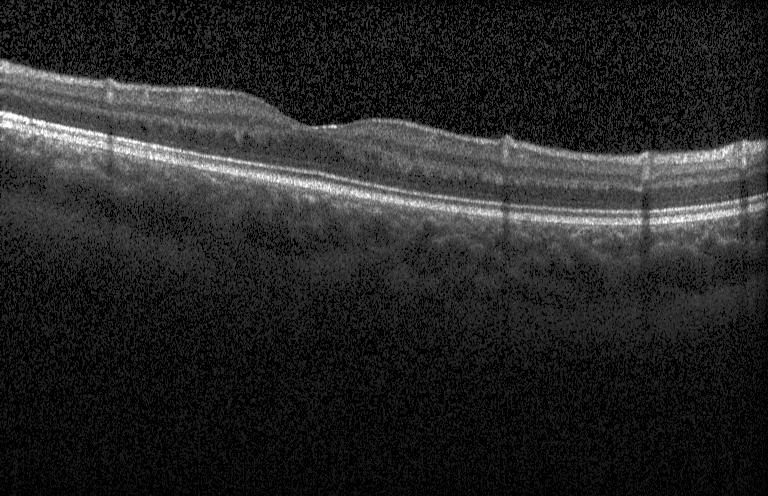 Horizontal scan through the fovea, optical coherence tomography scan.
Impression: no choroidal neovascularization, no diabetic macular edema, and no drusen.